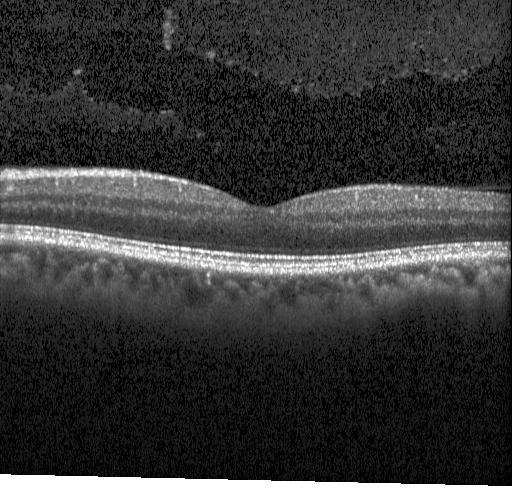 Optical coherence tomography scan · macular scan.
Diagnosis: no CNV, DME, or drusen.